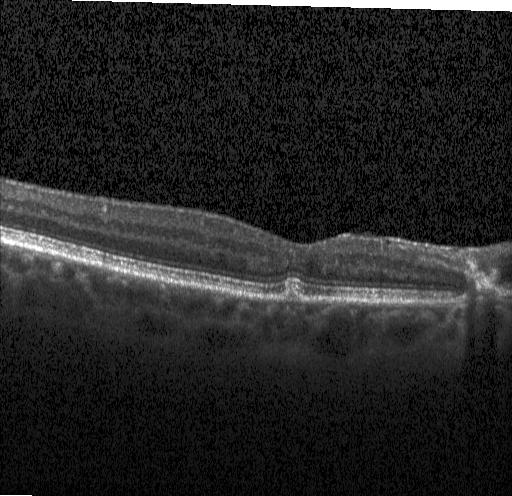
Impression: multiple drusen.